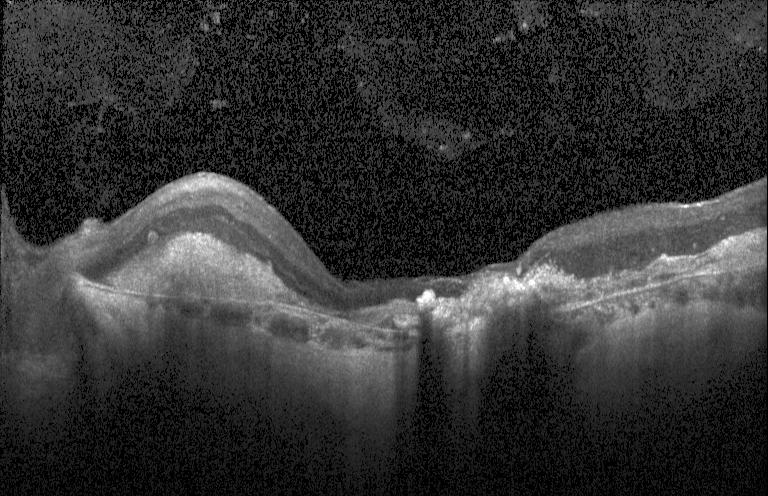
OCT B-scan, spectral-domain optical coherence tomography, through the macula. Diagnosis: choroidal neovascularization.